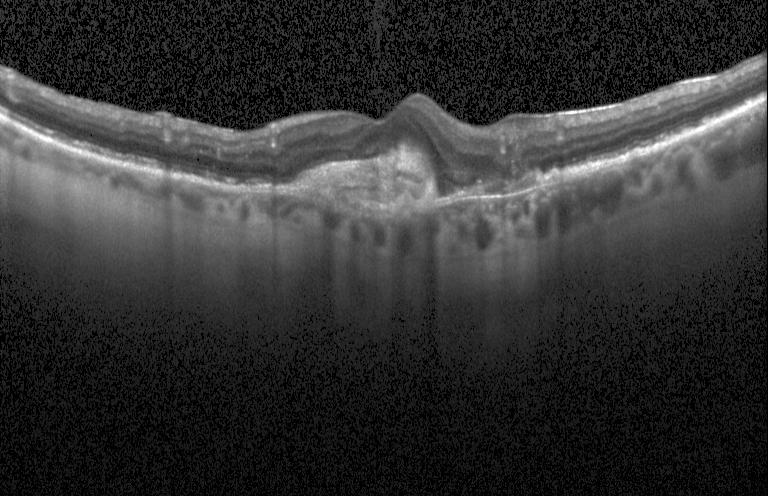

CNV.